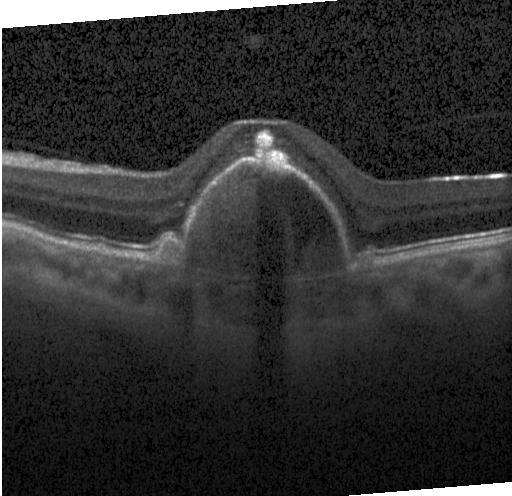 Optical coherence tomography B-scan
This B-scan demonstrates a choroidal neovascular membrane.